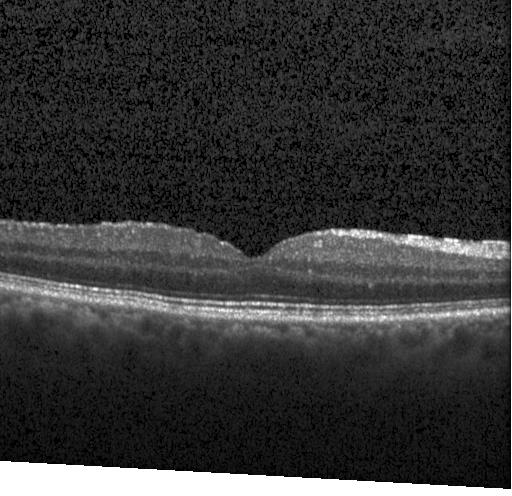
Impression: no CNV, no DME, and no drusen.